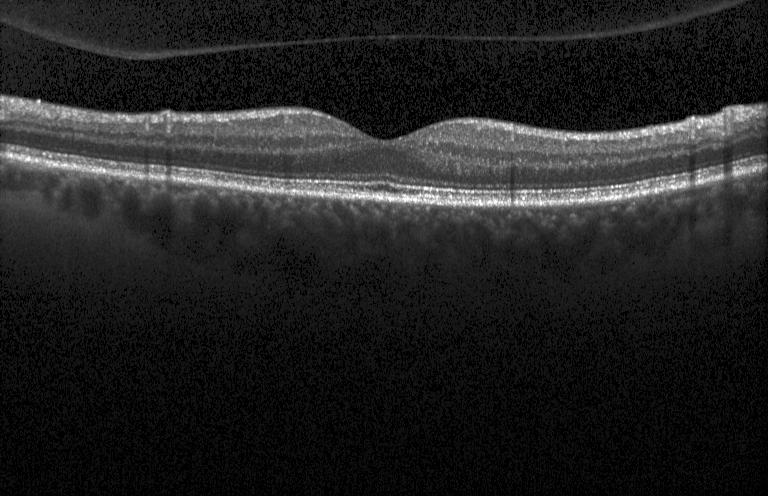 Acquired on a Heidelberg Spectralis. SD-OCT. OCT B-scan — Impression: neither choroidal neovascularization, diabetic macular edema, nor drusen.